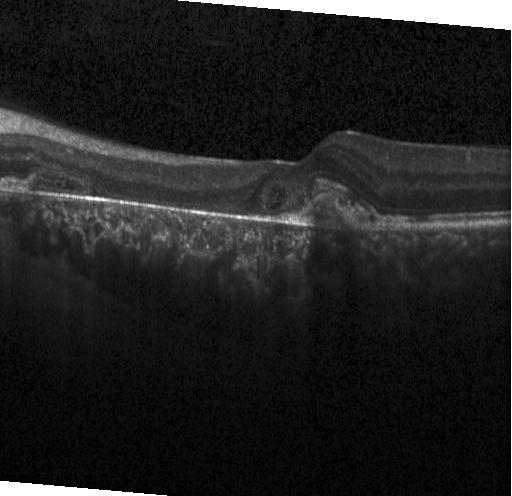 OCT B-scan. Centered on the fovea. Heidelberg Spectralis
Assessment: a choroidal neovascular membrane.